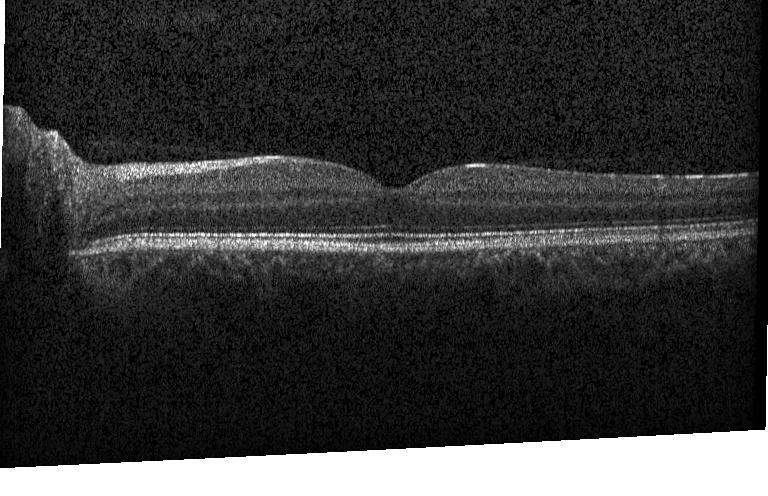
Finding: no CNV, no DME, and no drusen.